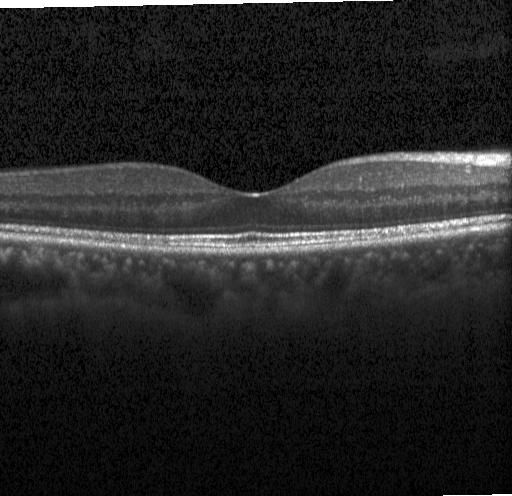 OCT line scan; SD-OCT; Heidelberg Spectralis OCT system
The scan shows no evidence of CNV, DME, or drusen.